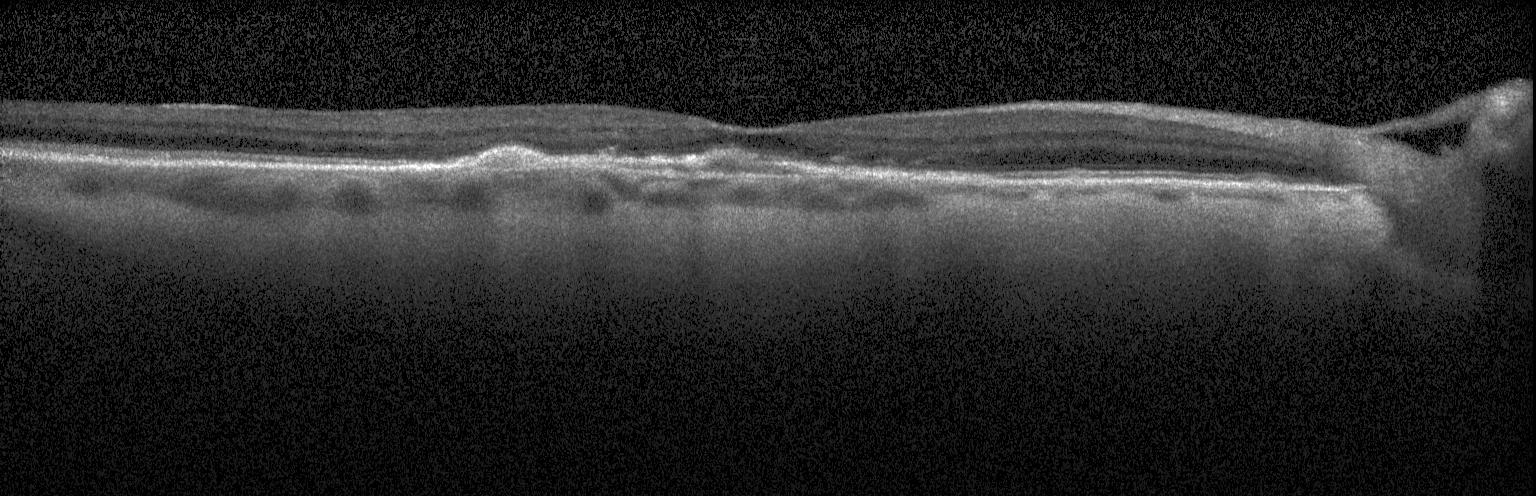 Heidelberg Spectralis OCT system, spectral-domain optical coherence tomography, horizontal scan through the fovea, optical coherence tomography scan. Diagnosis: a choroidal neovascular membrane.